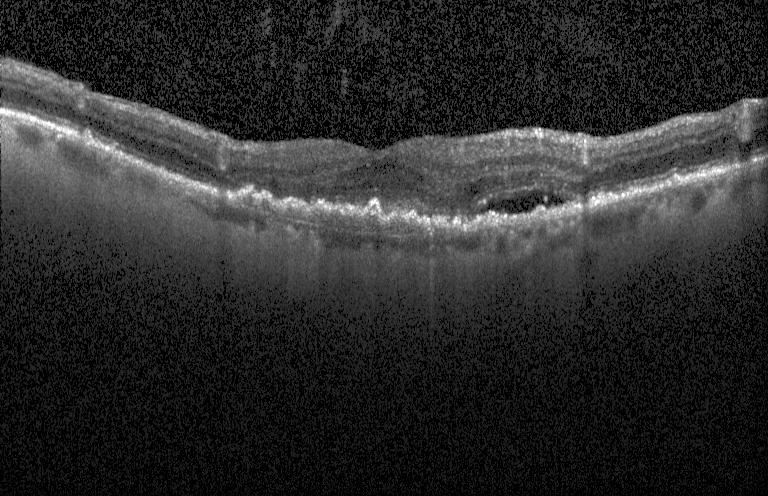

Instrument: Heidelberg Spectralis, OCT B-scan
Assessment: CNV.